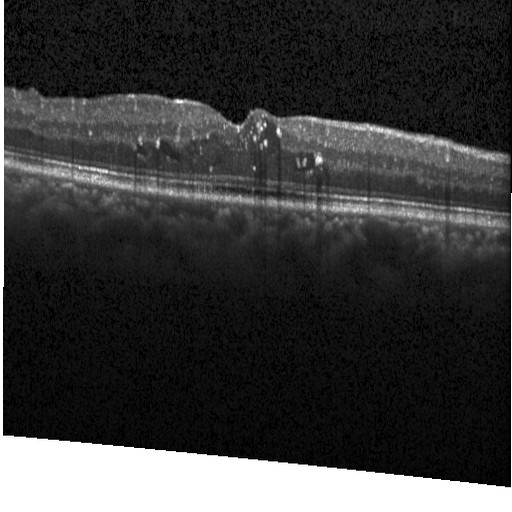 Optical coherence tomography scan; instrument: Heidelberg Spectralis; centered on the fovea; spectral-domain optical coherence tomography. Diabetic macular edema (DME).